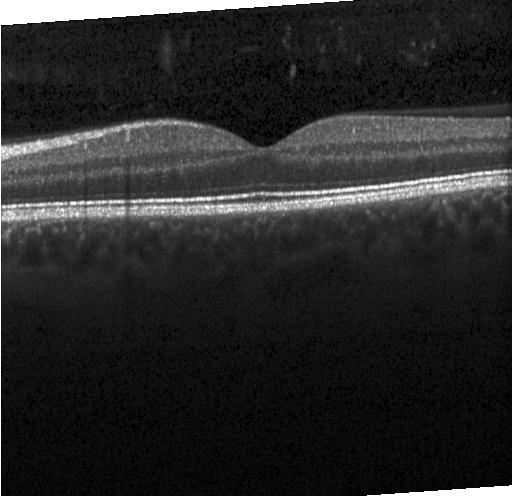 Fovea-centered, OCT line scan, Heidelberg Spectralis, spectral-domain OCT — The scan shows no evidence of choroidal neovascularization, diabetic macular edema, or drusen.